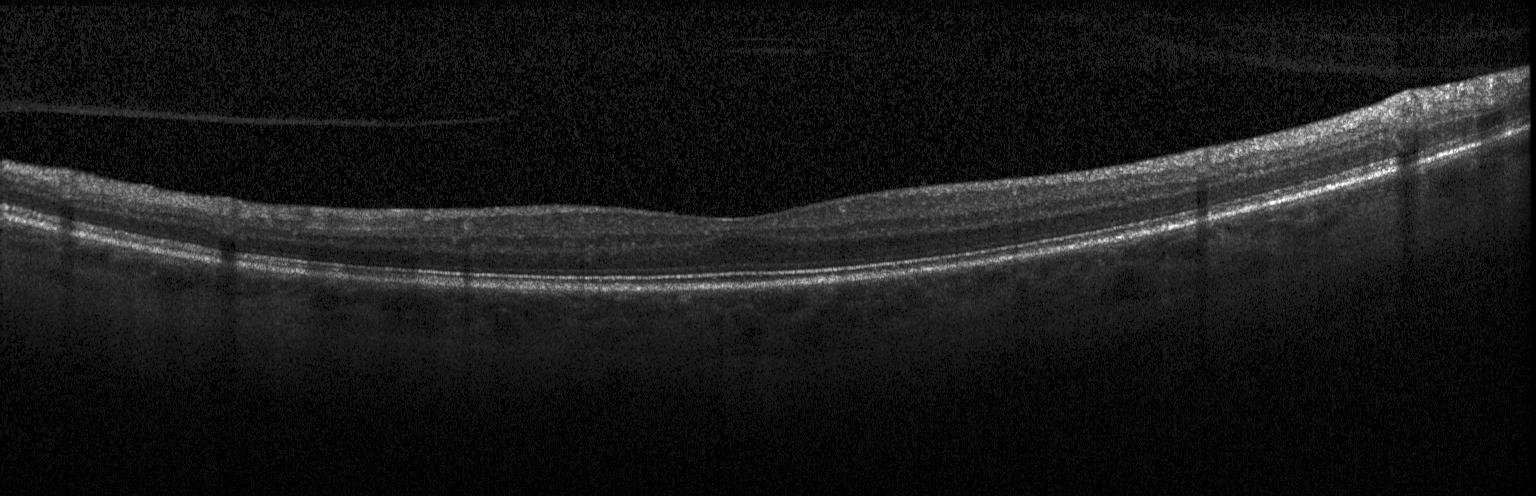

Spectral-domain OCT · optical coherence tomography scan · instrument: Heidelberg Spectralis · through the macula.
No evidence of choroidal neovascularization, diabetic macular edema, or drusen.